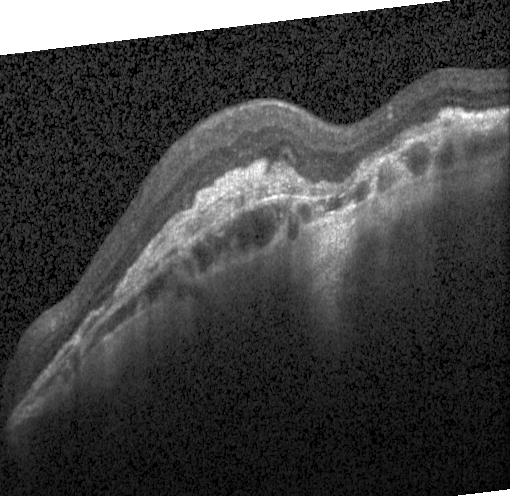 Through the macula, Heidelberg Spectralis OCT system, spectral-domain OCT, OCT B-scan.
Impression: choroidal neovascularization (CNV).